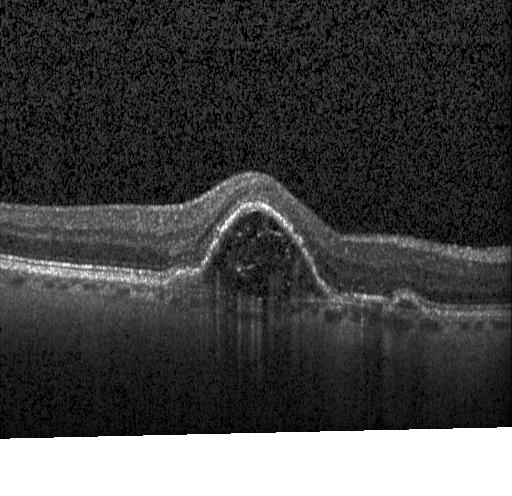
OCT finding: choroidal neovascularization (CNV).